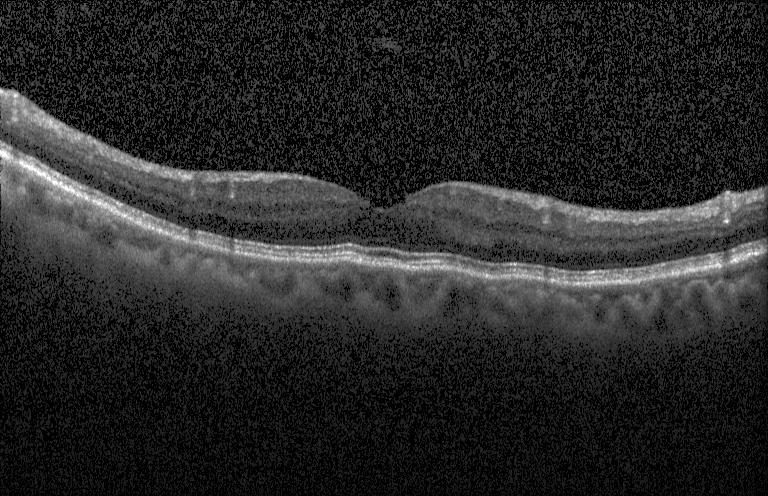

Acquired on a Heidelberg Spectralis · OCT B-scan.
Finding: no evidence of choroidal neovascularization, diabetic macular edema, or drusen.